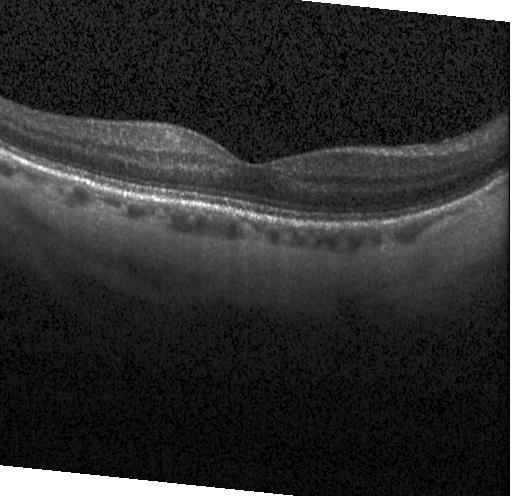

Retinal OCT B-scan
Impression: no evidence of choroidal neovascularization, diabetic macular edema, or drusen.